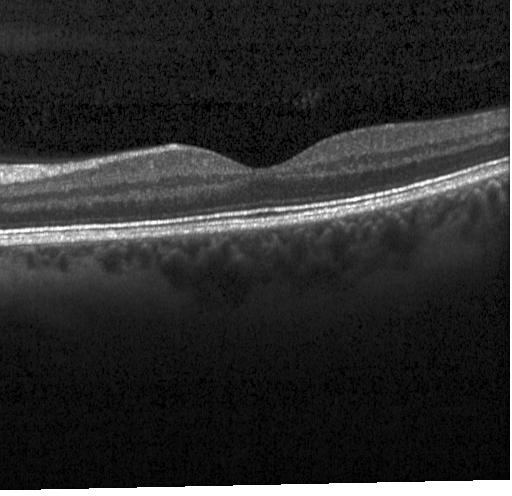 Assessment: no evidence of choroidal neovascularization, diabetic macular edema, or drusen.